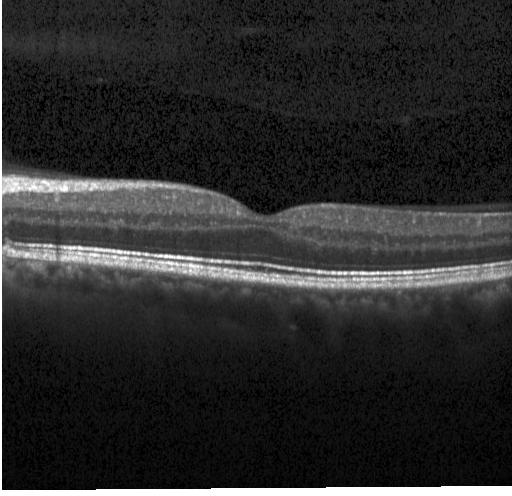

OCT line scan; Heidelberg Spectralis OCT system; centered on the fovea — Assessment: no evidence of choroidal neovascularization, diabetic macular edema, or drusen.